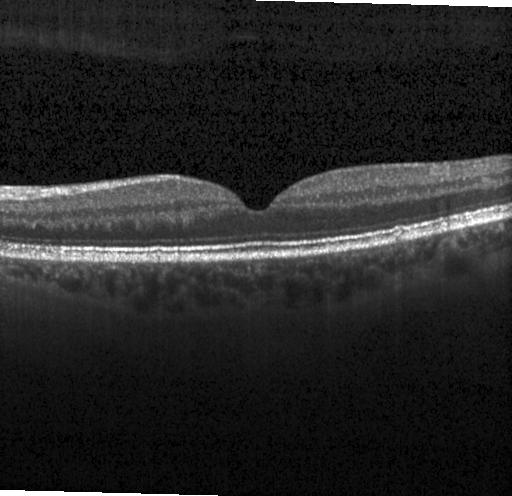
Finding: no choroidal neovascularization, no diabetic macular edema, and no drusen.